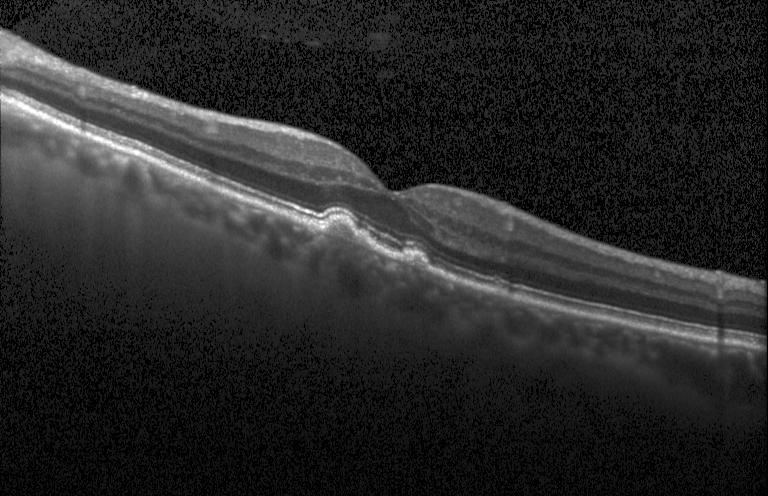
Retinal OCT cross-section. Instrument: Heidelberg Spectralis
Assessment: multiple drusen.